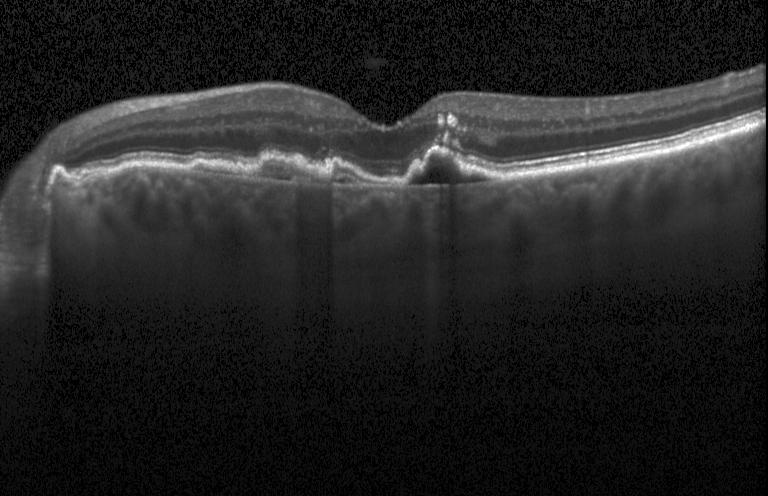
Centered on the fovea. SD-OCT. Heidelberg Spectralis OCT system. OCT B-scan
Dx: choroidal neovascularization (CNV).